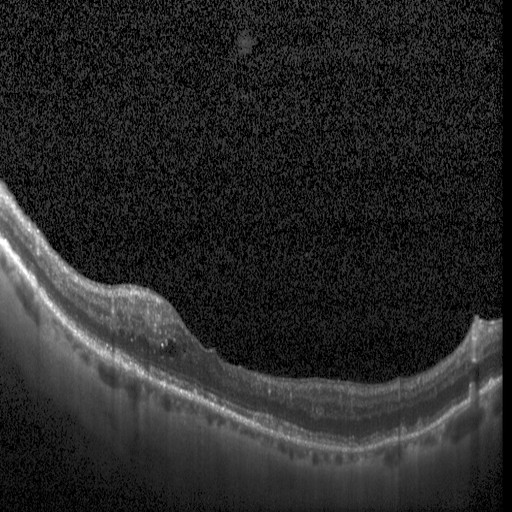 OCT B-scan — OCT finding: diabetic macular edema (DME).